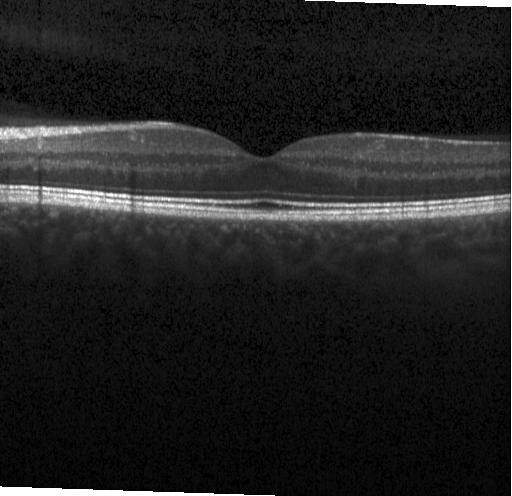 OCT line scan.
OCT finding: no CNV, no DME, and no drusen.